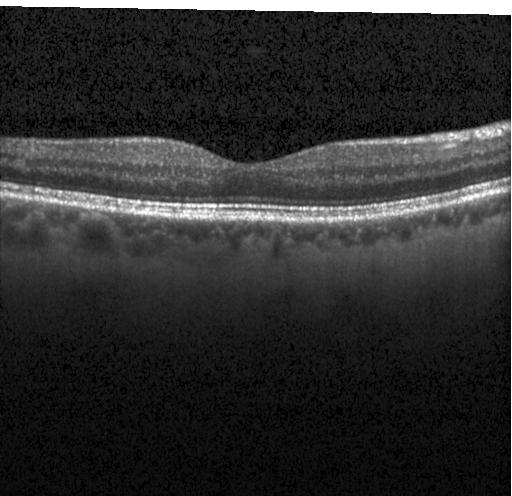 OCT B-scan showing no choroidal neovascularization, no diabetic macular edema, and no drusen.